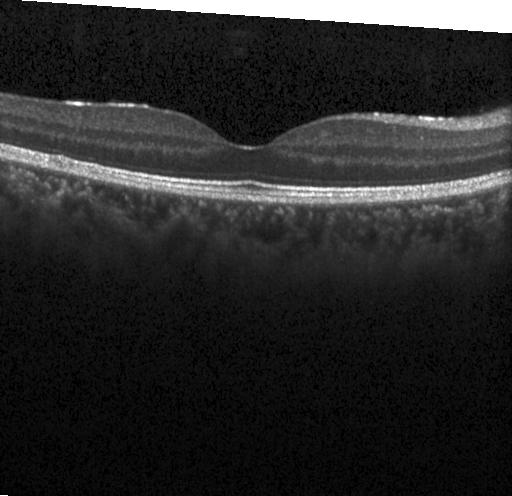

Heidelberg Spectralis, OCT line scan. Finding: no evidence of choroidal neovascularization, diabetic macular edema, or drusen.